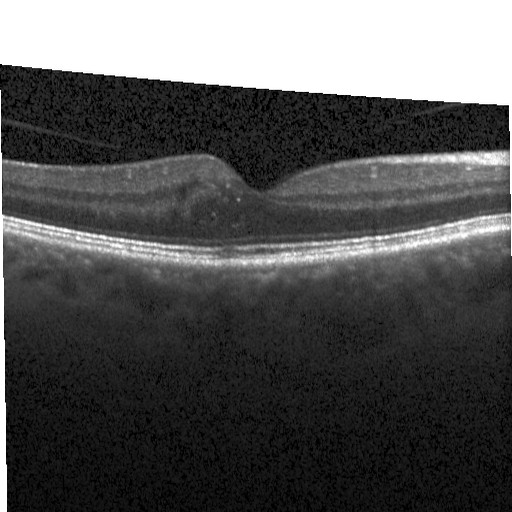 Horizontal scan through the fovea; retinal OCT B-scan. Impression: diabetic macular edema (DME).